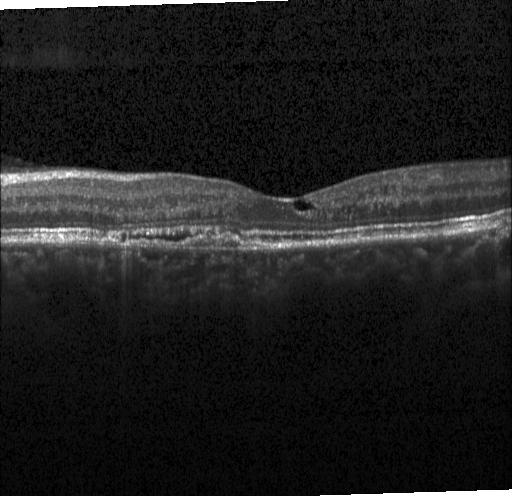

This B-scan demonstrates CNV.